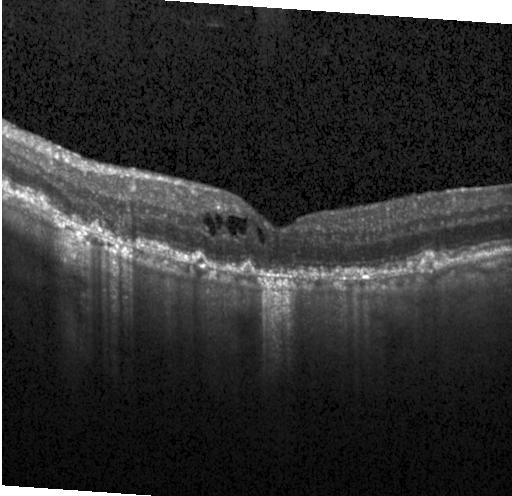
Optical coherence tomography B-scan.
Dx: a choroidal neovascular membrane.